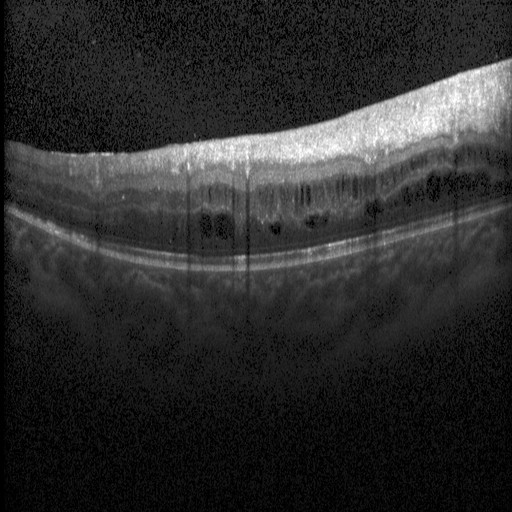

Retinal OCT cross-section showing diabetic macular edema.